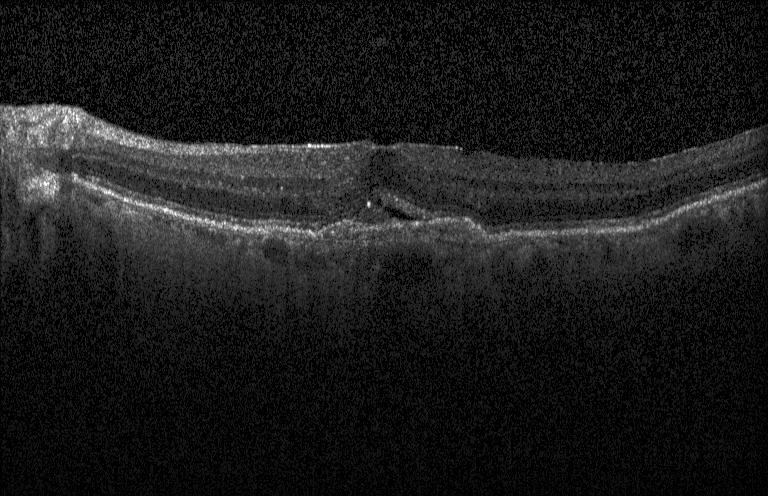 Macular scan; retinal OCT cross-section
Assessment: a choroidal neovascular membrane.